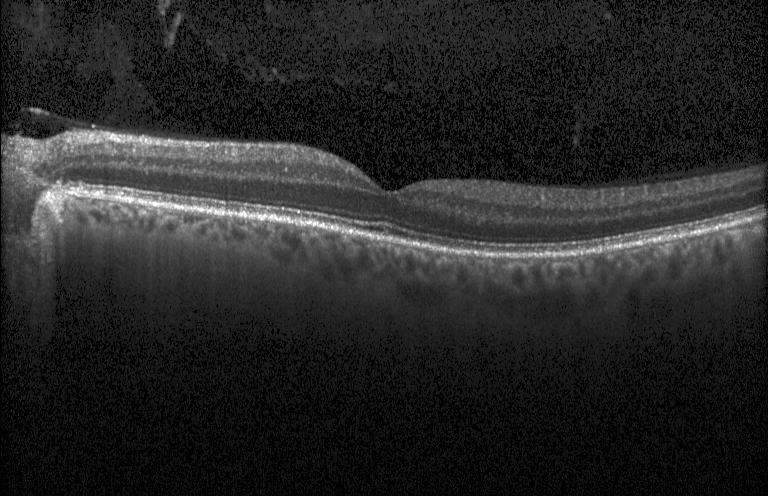
The scan shows neither choroidal neovascularization, diabetic macular edema, nor drusen.